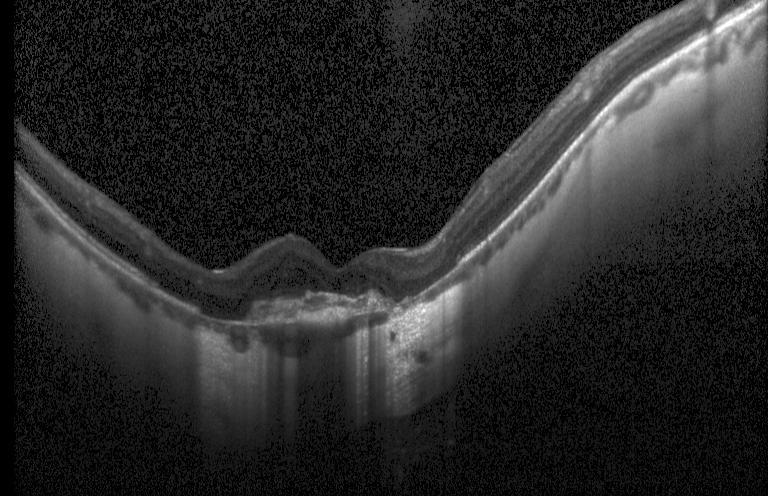
OCT finding: a choroidal neovascular membrane.